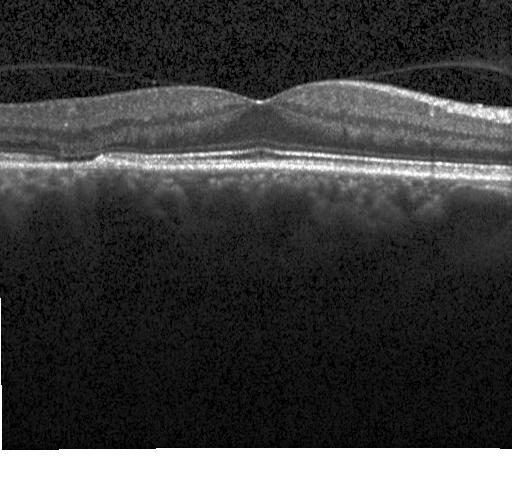
OCT B-scan. Finding: a choroidal neovascular membrane.